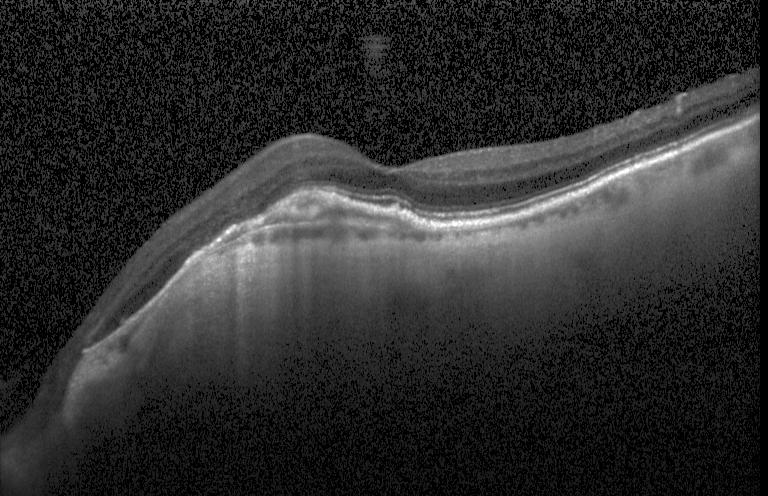
OCT scan showing a choroidal neovascular membrane.